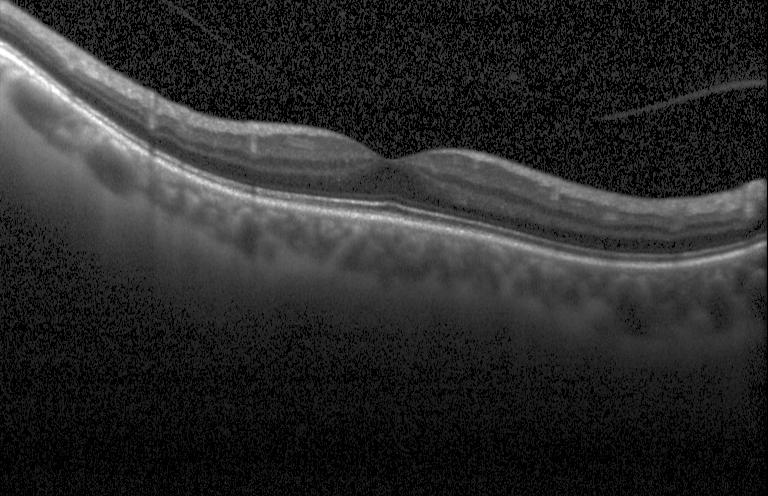
Heidelberg Spectralis. Macular scan. OCT line scan — Diagnosis: neither choroidal neovascularization, diabetic macular edema, nor drusen.